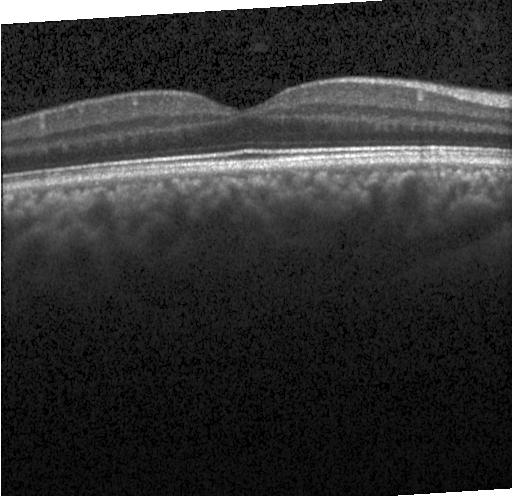
Retinal OCT cross-section showing no evidence of choroidal neovascularization, diabetic macular edema, or drusen.